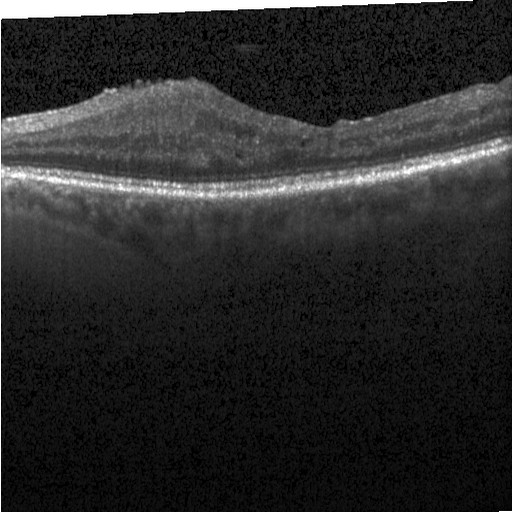 Finding: diabetic macular edema (DME).